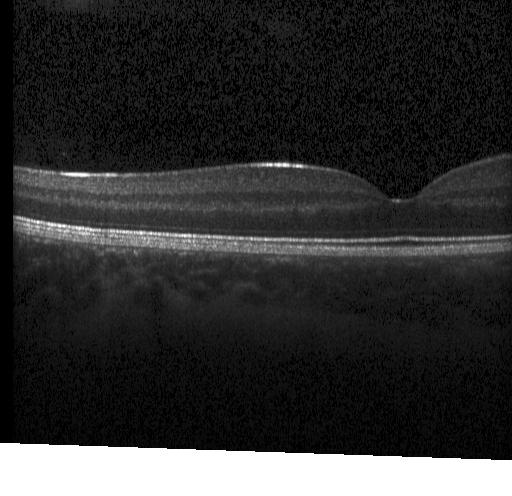
Centered on the fovea. Retinal OCT cross-section.
Diagnosis: no evidence of choroidal neovascularization, diabetic macular edema, or drusen.